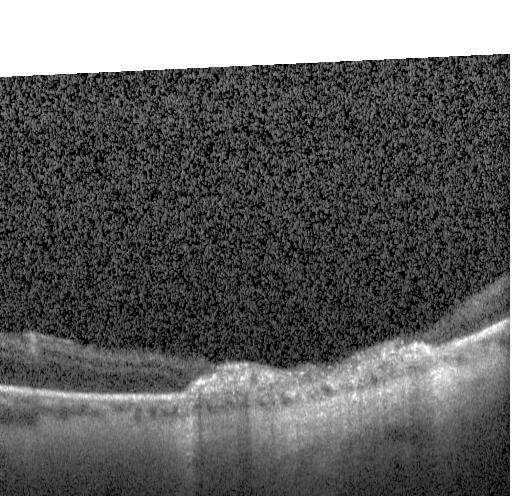 OCT B-scan, instrument: Heidelberg Spectralis, SD-OCT.
Dx: a choroidal neovascular membrane.